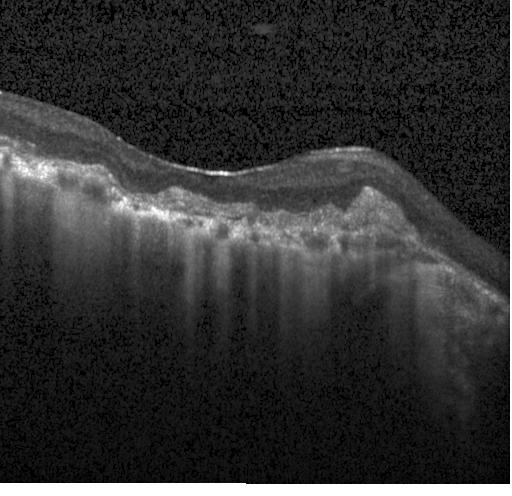 Optical coherence tomography B-scan. Spectral-domain OCT — Dx: a choroidal neovascular membrane.